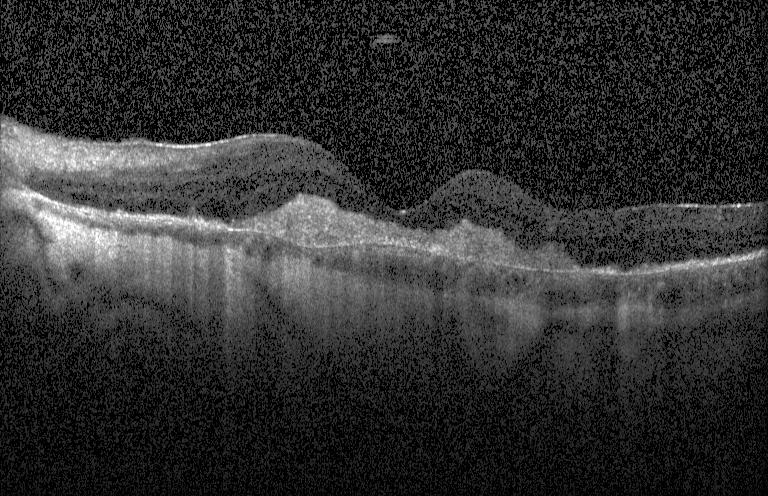

Macular OCT demonstrating a choroidal neovascular membrane.